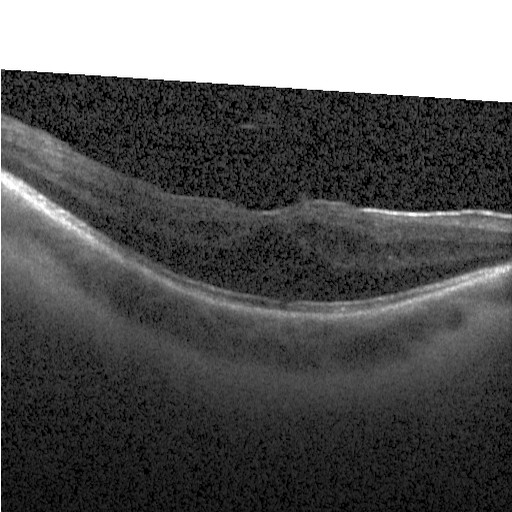 Heidelberg Spectralis OCT system; optical coherence tomography scan; through the macula; SD-OCT
Dx: diabetic macular edema.